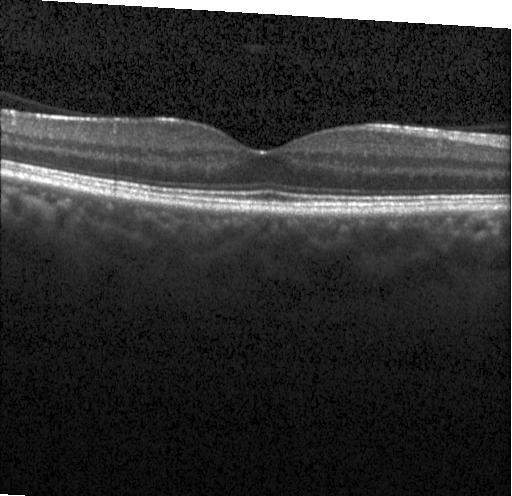

Macular OCT demonstrating neither CNV, DME, nor drusen.